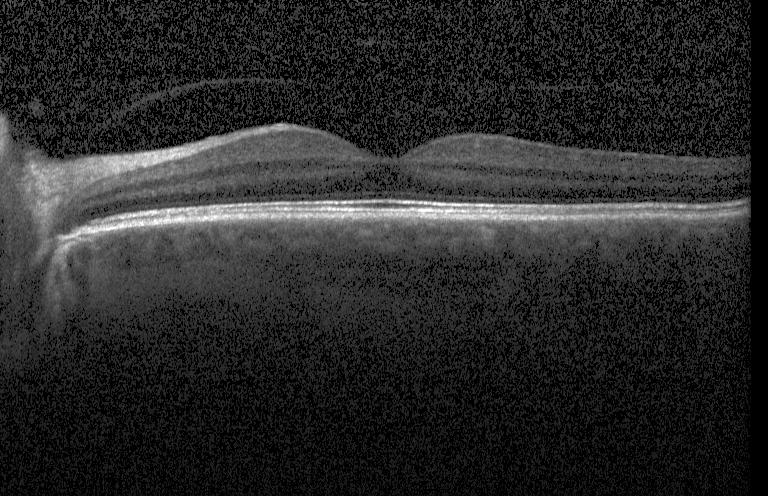
Retinal OCT B-scan · acquired on a Heidelberg Spectralis — Impression: no choroidal neovascularization, no diabetic macular edema, and no drusen.